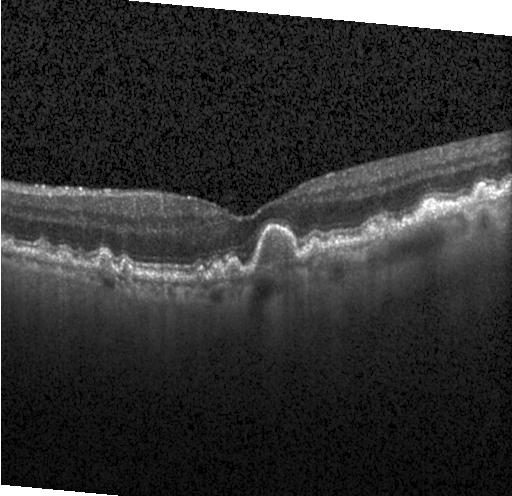
OCT line scan
OCT finding: multiple drusen.